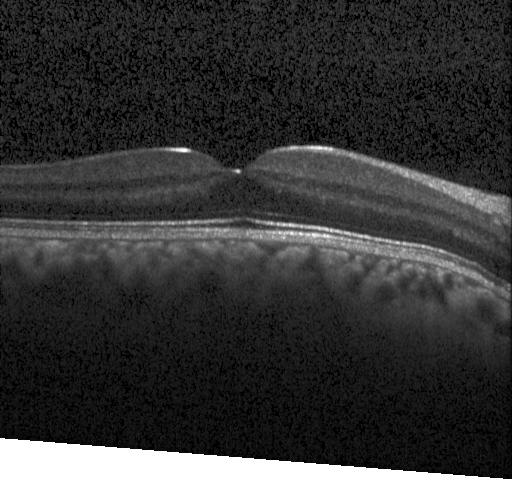 OCT B-scan showing no choroidal neovascularization, no diabetic macular edema, and no drusen.